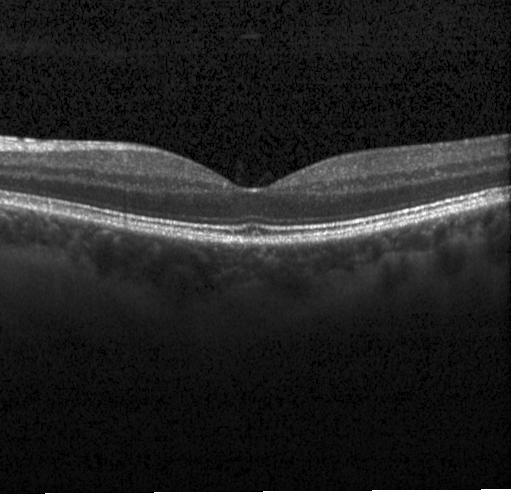 Retinal OCT B-scan
Diagnosis: neither CNV, DME, nor drusen.